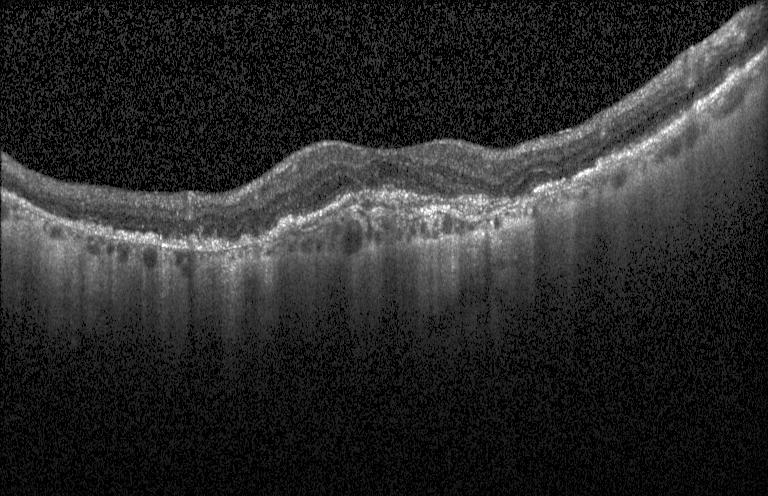 OCT line scan, centered on the fovea. Macular OCT: a choroidal neovascular membrane.